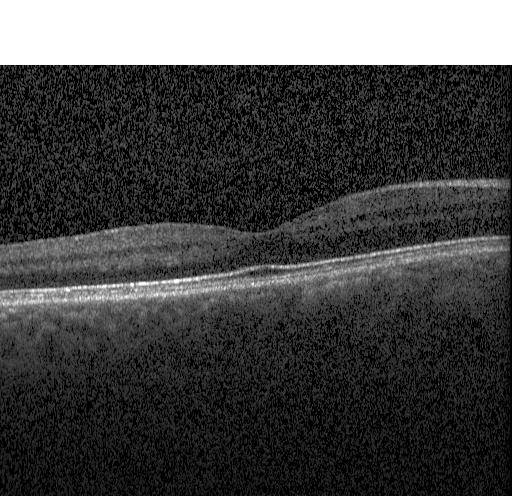

Retinal OCT B-scan
Assessment: no choroidal neovascularization, no diabetic macular edema, and no drusen.